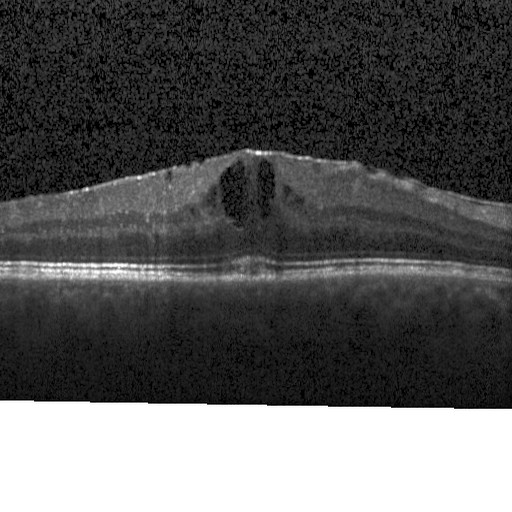
SD-OCT; optical coherence tomography B-scan; centered on the fovea; instrument: Heidelberg Spectralis.
Macular OCT: diabetic macular edema (DME).